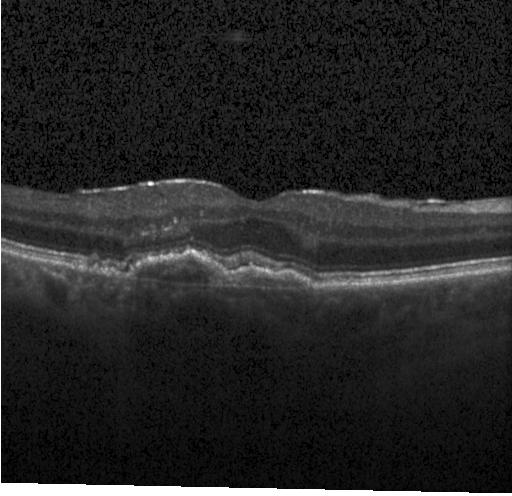

OCT finding: a choroidal neovascular membrane.